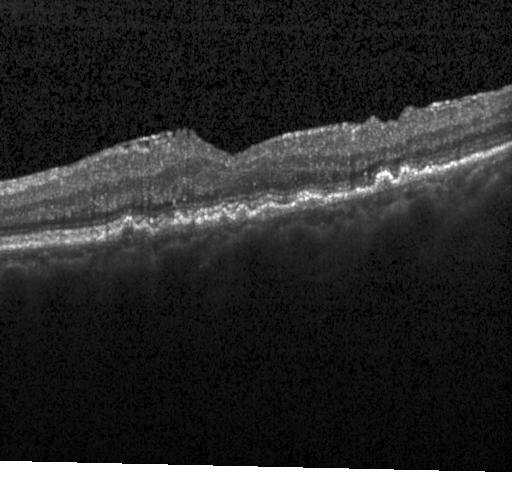
Retinal OCT cross-section · Heidelberg Spectralis · centered on the fovea.
Finding: sub-RPE drusenoid deposits.